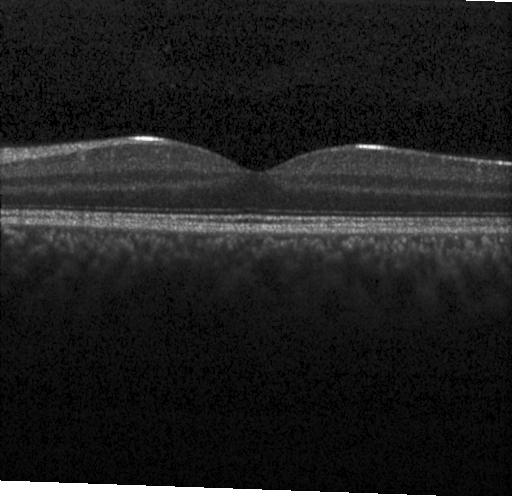

Macular OCT: neither choroidal neovascularization, diabetic macular edema, nor drusen.